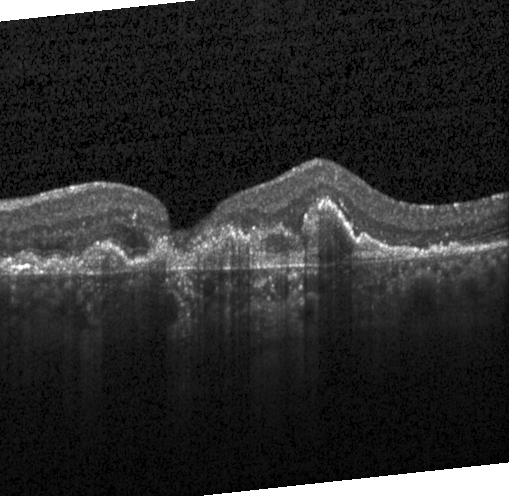
Optical coherence tomography scan · macular scan — OCT finding: CNV.